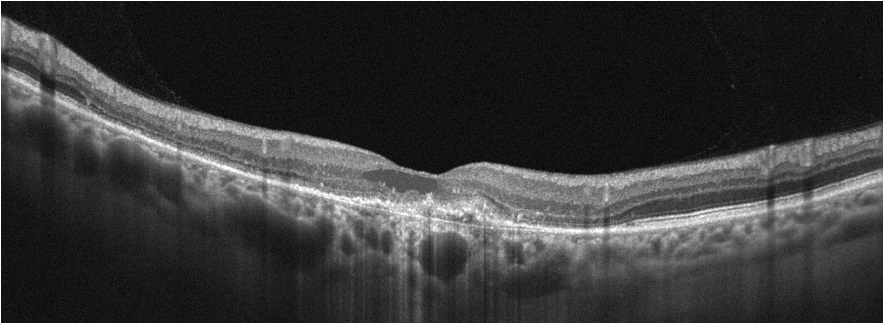
Impression: AMD.